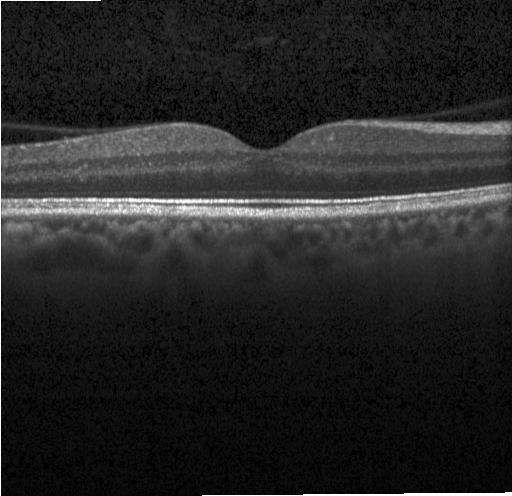 OCT B-scan — Finding: neither choroidal neovascularization, diabetic macular edema, nor drusen.